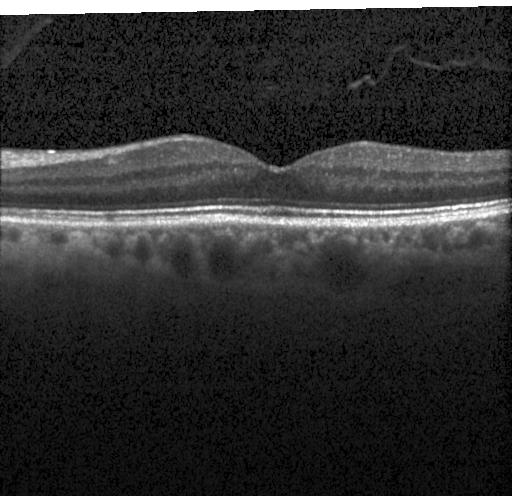

Heidelberg Spectralis OCT system. Optical coherence tomography B-scan. Spectral-domain OCT
Impression: no evidence of CNV, DME, or drusen.